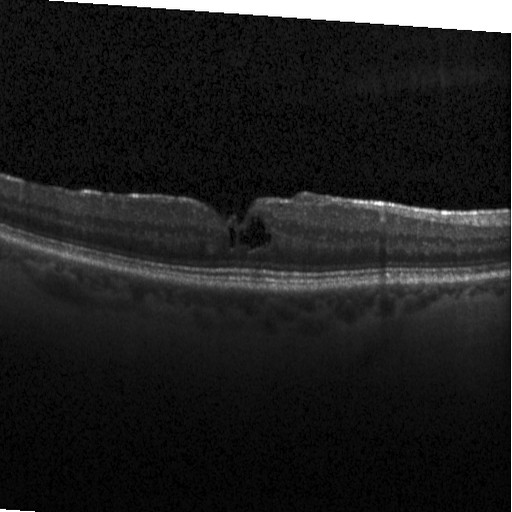
Diagnosis: diabetic macular edema (DME).